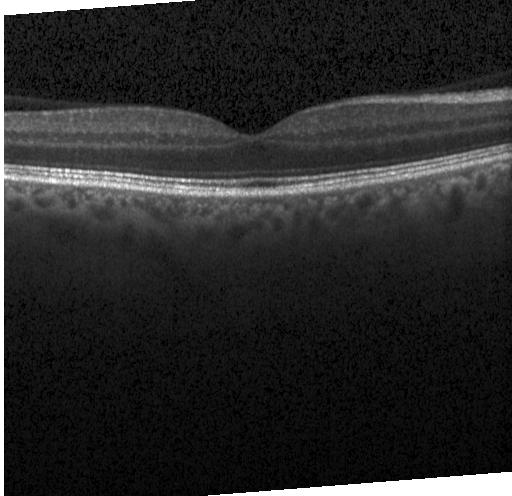
Retinal OCT B-scan; spectral-domain optical coherence tomography — Impression: no CNV, no DME, and no drusen.